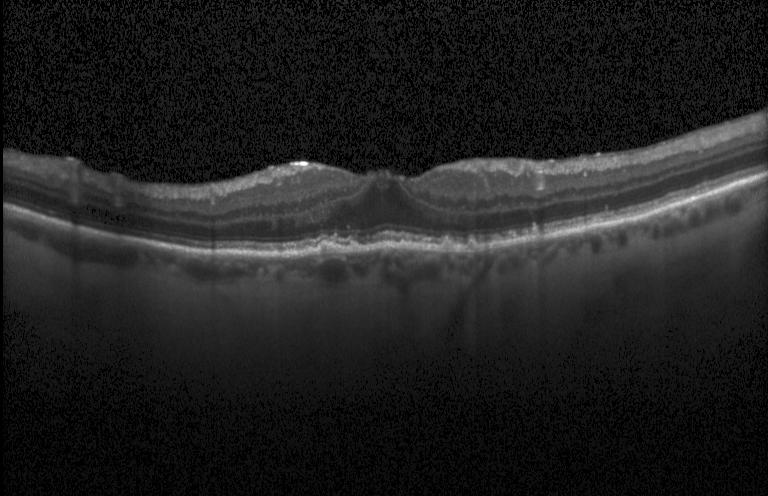 Centered on the fovea. Instrument: Heidelberg Spectralis. OCT B-scan — Dx: sub-RPE drusenoid deposits.